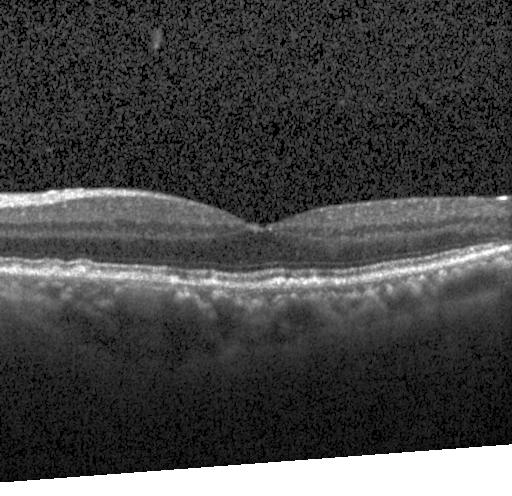 Sub-RPE drusenoid deposits.